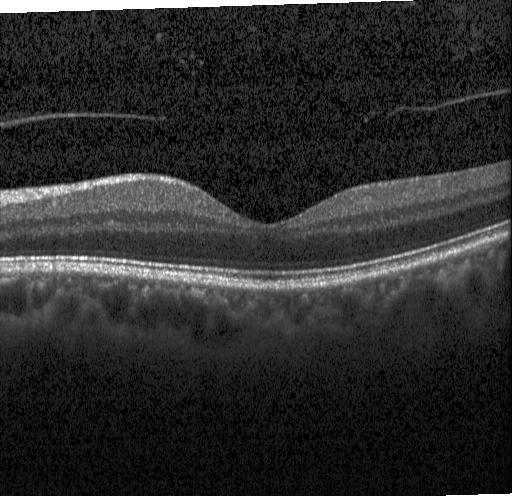

Optical coherence tomography B-scan; spectral-domain optical coherence tomography; instrument: Heidelberg Spectralis; horizontal scan through the fovea.
The scan shows neither CNV, DME, nor drusen.